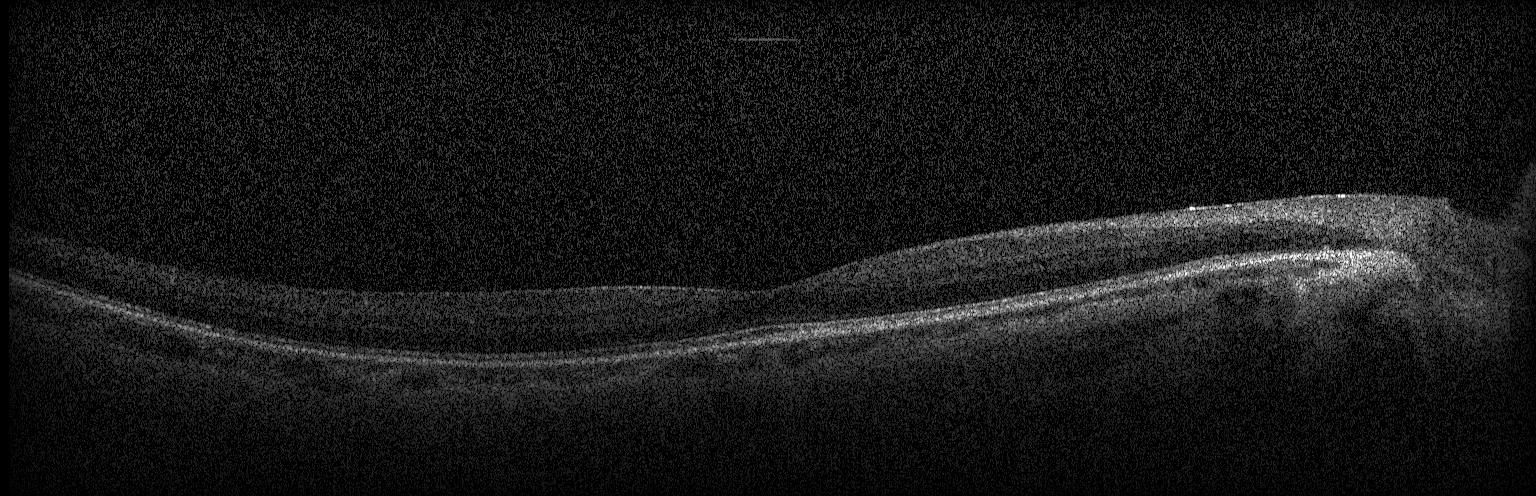
OCT B-scan showing no choroidal neovascularization, diabetic macular edema, or drusen.